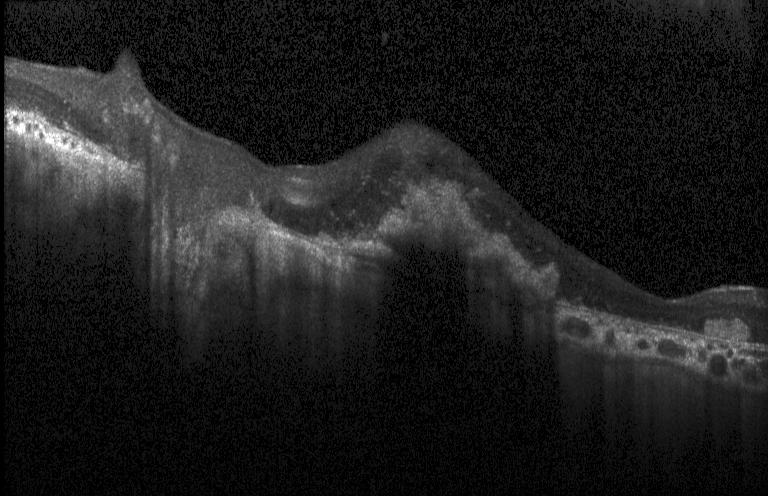

OCT B-scan. Instrument: Heidelberg Spectralis.
Impression: choroidal neovascularization (CNV).